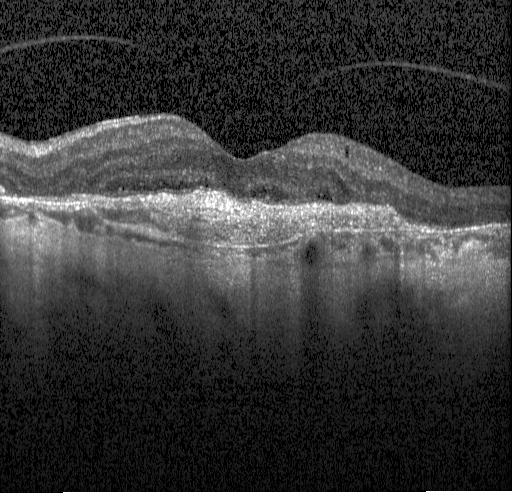
Diagnosis: a choroidal neovascular membrane.